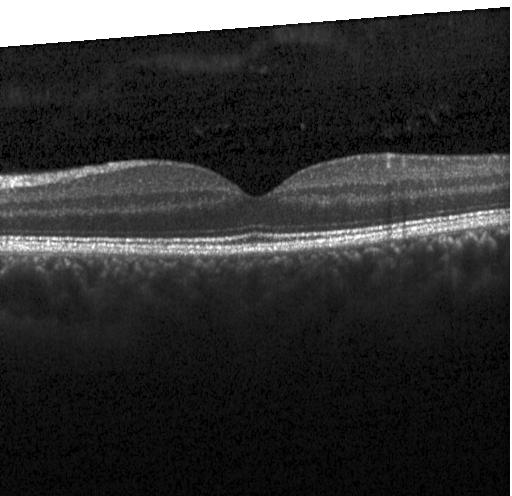
Centered on the fovea · optical coherence tomography scan. Dx: no choroidal neovascularization, no diabetic macular edema, and no drusen.